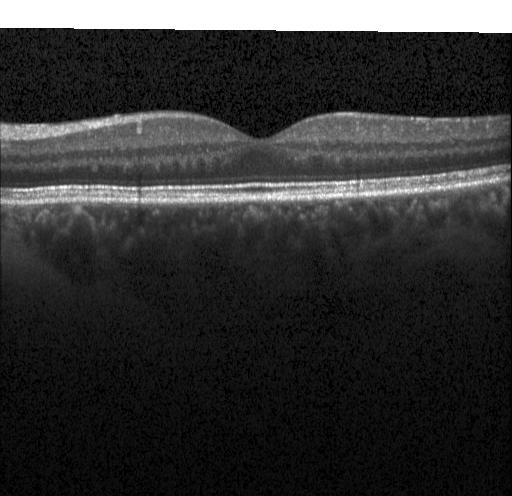 Impression: no evidence of choroidal neovascularization, diabetic macular edema, or drusen.